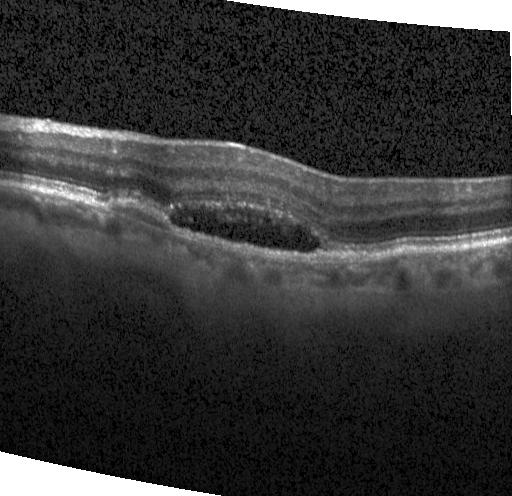
Optical coherence tomography B-scan
Diagnosis: a choroidal neovascular membrane.